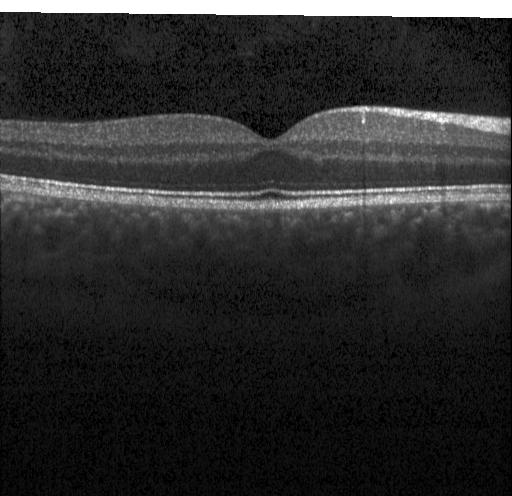

Impression: no evidence of choroidal neovascularization, diabetic macular edema, or drusen.